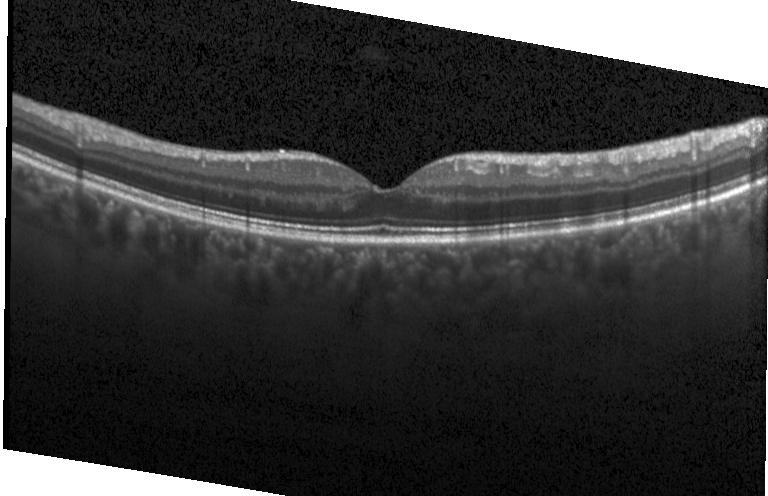
Spectral-domain optical coherence tomography · centered on the fovea · retinal OCT B-scan · Heidelberg Spectralis. Dx: no choroidal neovascularization, diabetic macular edema, or drusen.